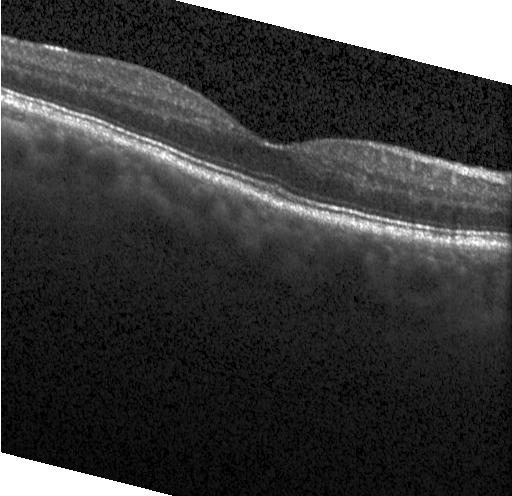 OCT line scan — Finding: no choroidal neovascularization, diabetic macular edema, or drusen.